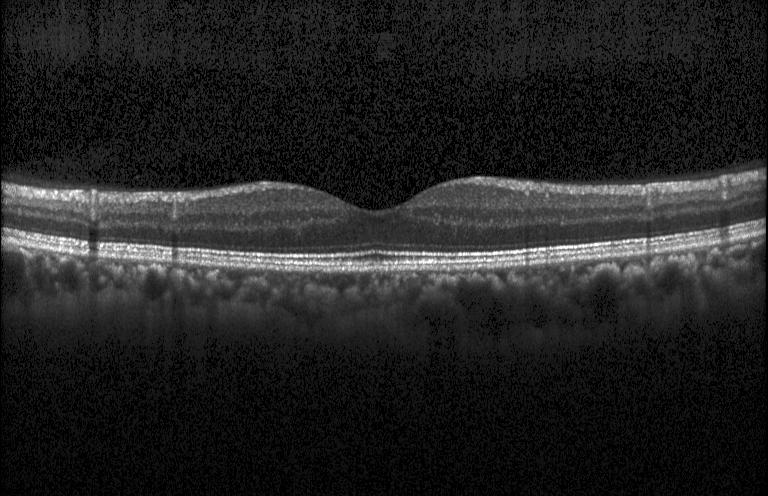
This B-scan demonstrates no choroidal neovascularization, no diabetic macular edema, and no drusen.